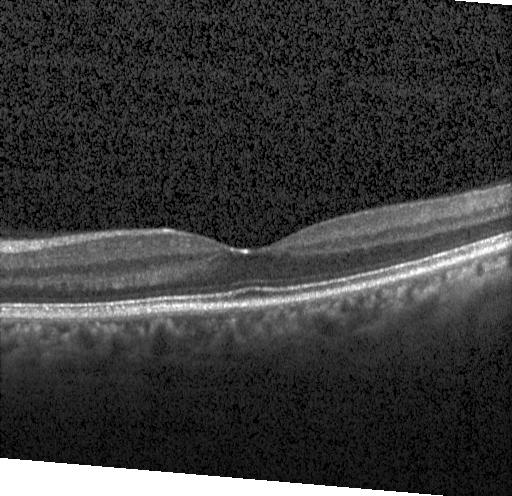 Optical coherence tomography B-scan. SD-OCT. Fovea-centered.
Finding: no choroidal neovascularization, no diabetic macular edema, and no drusen.